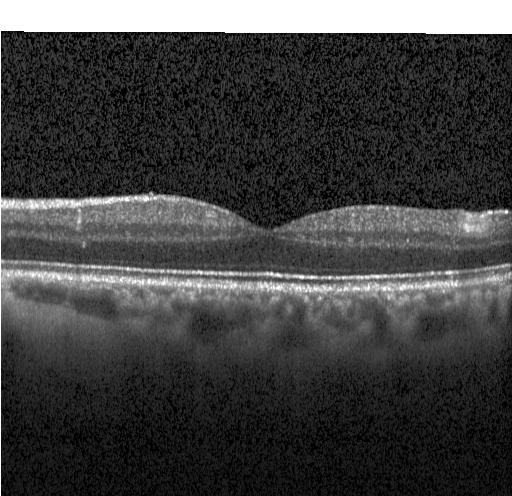
Retinal OCT B-scan.
Finding: neither choroidal neovascularization, diabetic macular edema, nor drusen.